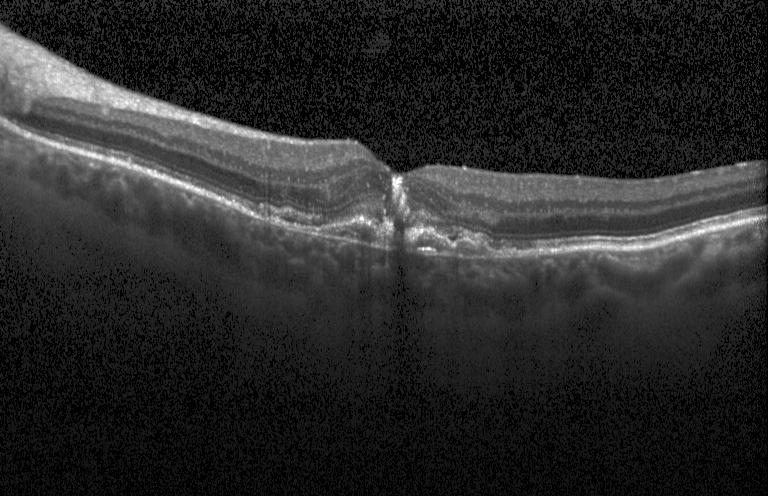

Heidelberg Spectralis OCT system; OCT B-scan.
Finding: choroidal neovascularization (CNV).